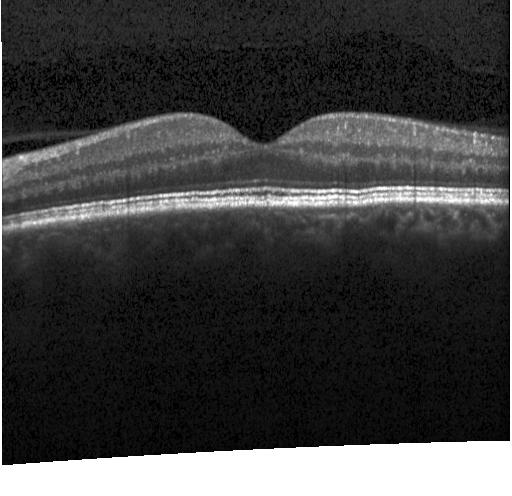
OCT line scan.
Impression: neither choroidal neovascularization, diabetic macular edema, nor drusen.